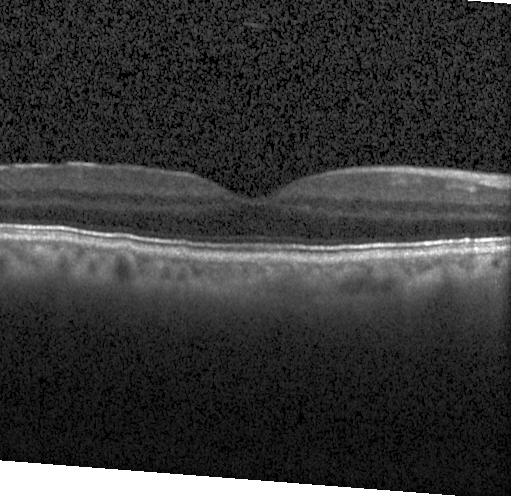
OCT line scan — Impression: neither CNV, DME, nor drusen.